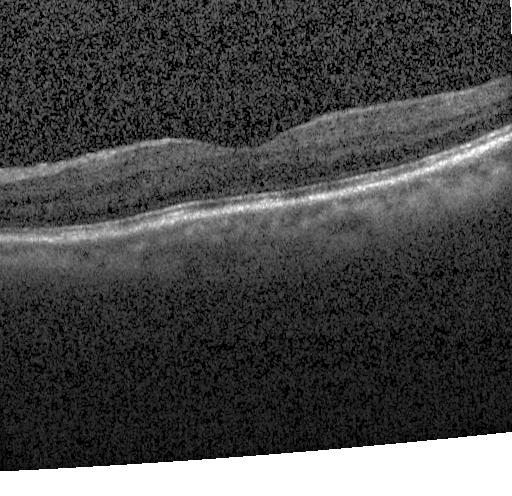
Horizontal scan through the fovea; retinal OCT cross-section; spectral-domain OCT.
Diagnosis: no CNV, DME, or drusen.